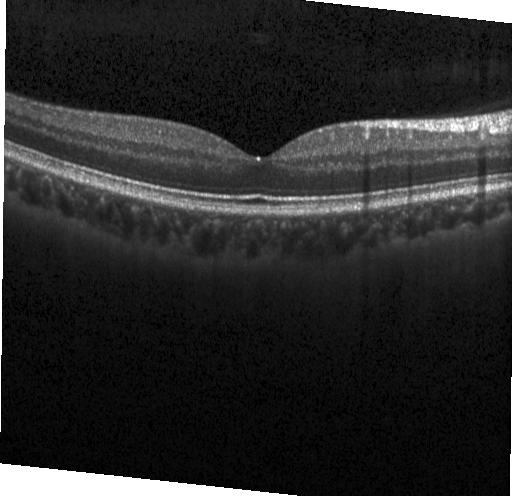
Instrument: Heidelberg Spectralis, centered on the fovea, spectral-domain optical coherence tomography, retinal OCT B-scan. This B-scan demonstrates neither CNV, DME, nor drusen.